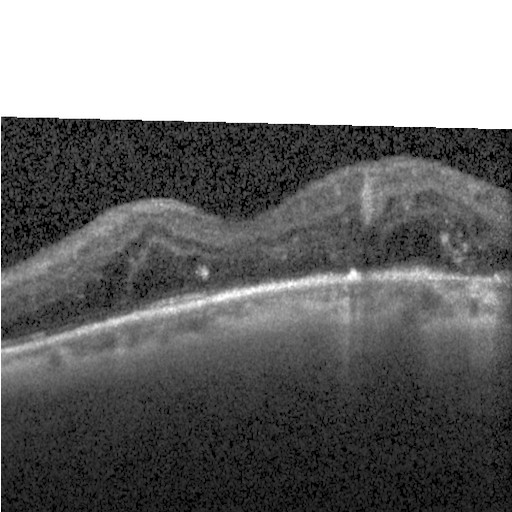

Diagnosis: DME.